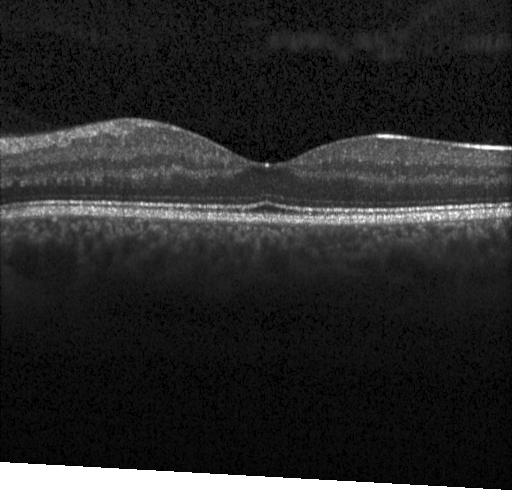

Retinal OCT cross-section showing no choroidal neovascularization, diabetic macular edema, or drusen.